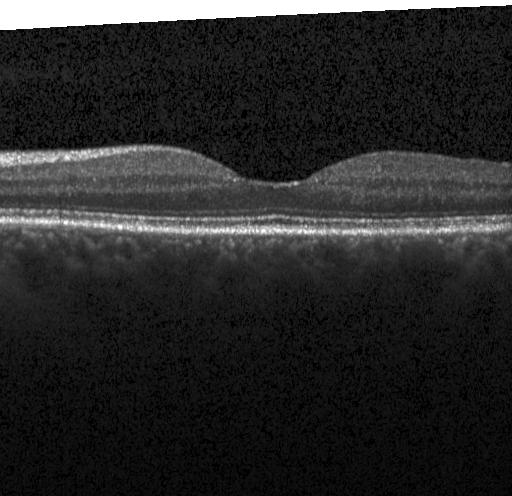 Optical coherence tomography B-scan. Heidelberg Spectralis. Spectral-domain OCT
Impression: no evidence of choroidal neovascularization, diabetic macular edema, or drusen.